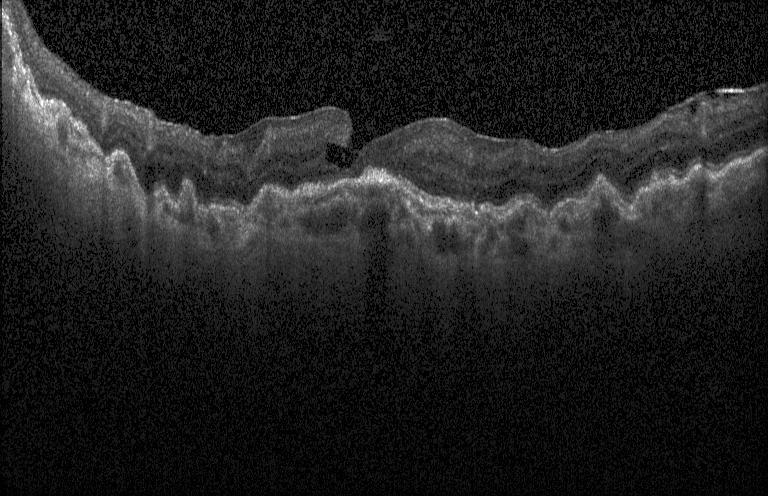

Optical coherence tomography scan, spectral-domain OCT.
Assessment: CNV.